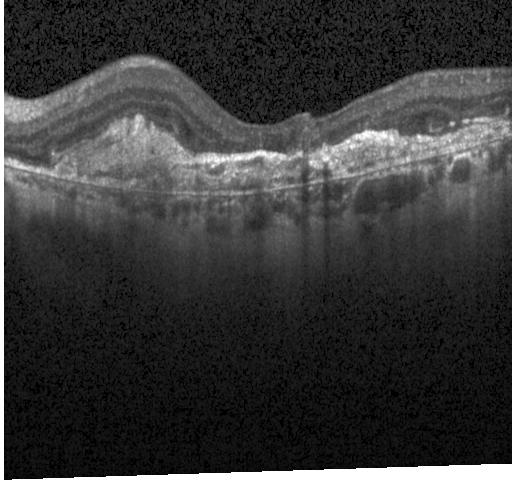

Macular scan. Spectral-domain optical coherence tomography. Retinal OCT cross-section.
Impression: CNV.